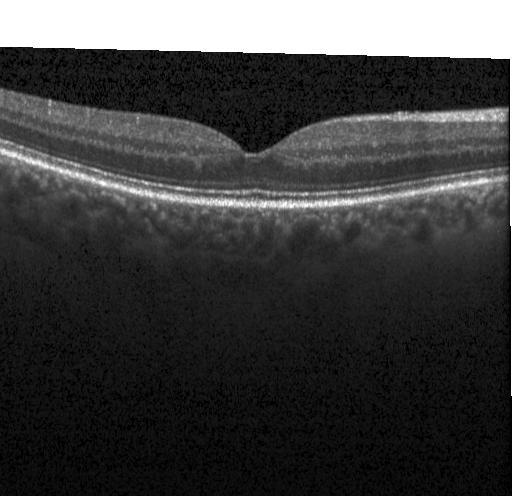
Impression: no evidence of CNV, DME, or drusen.